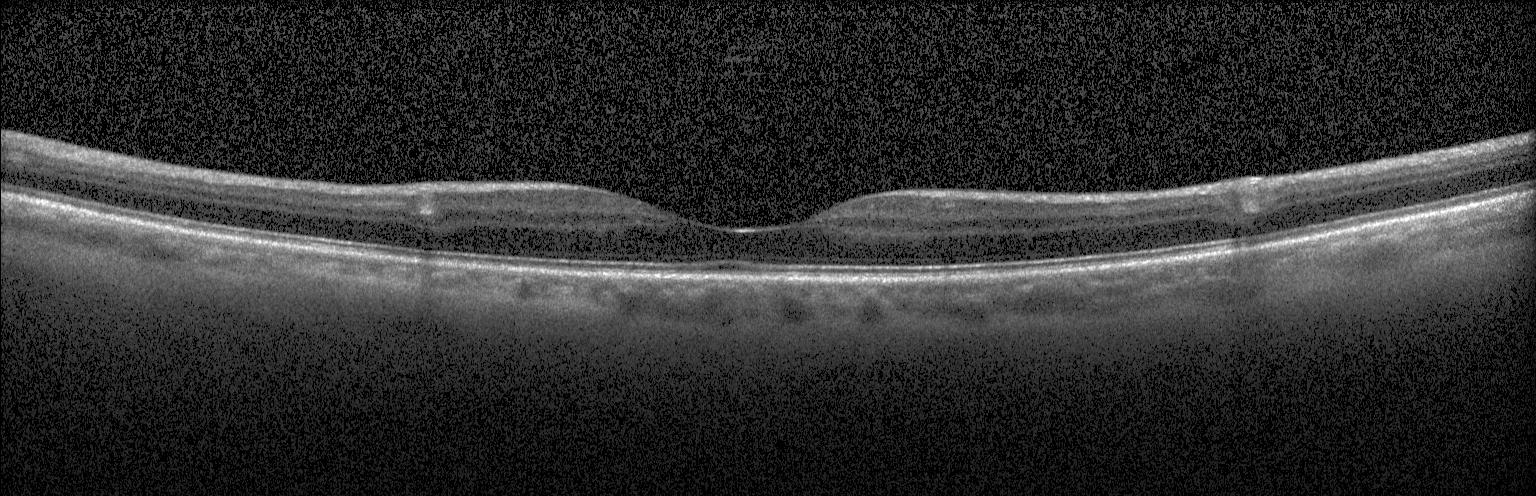

Retinal OCT B-scan.
Impression: neither choroidal neovascularization, diabetic macular edema, nor drusen.